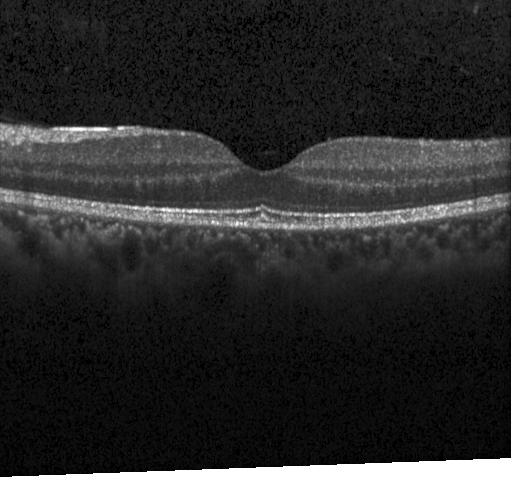 OCT B-scan. Spectral-domain OCT. Heidelberg Spectralis. Fovea-centered
No CNV, no DME, and no drusen.